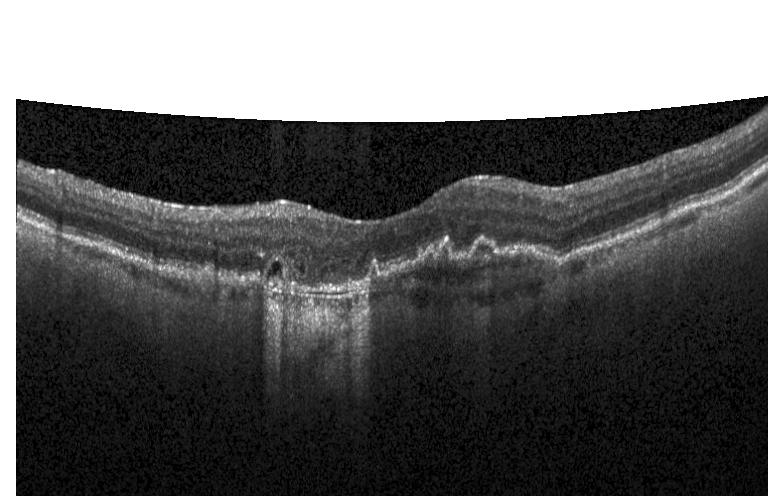
Spectral-domain optical coherence tomography; Heidelberg Spectralis; optical coherence tomography B-scan; centered on the fovea.
The scan shows choroidal neovascularization.